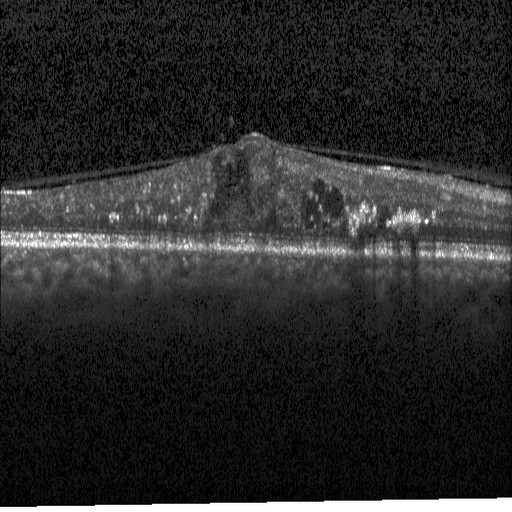
This B-scan demonstrates diabetic macular edema (DME).